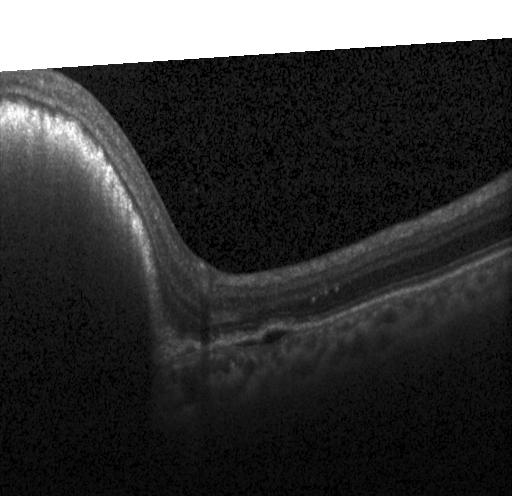

OCT line scan. The scan shows a choroidal neovascular membrane.